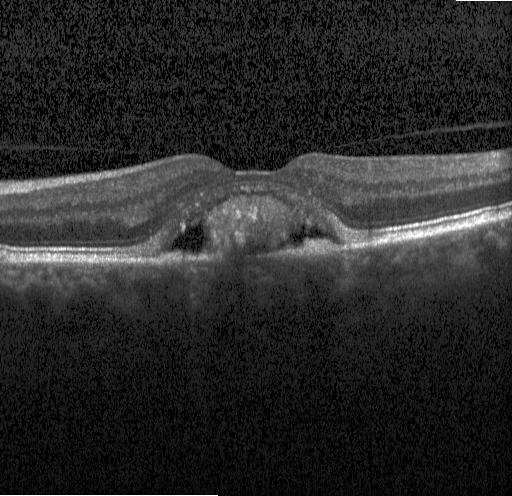
Retinal OCT B-scan · Heidelberg Spectralis OCT system · fovea-centered — Diagnosis: a choroidal neovascular membrane.